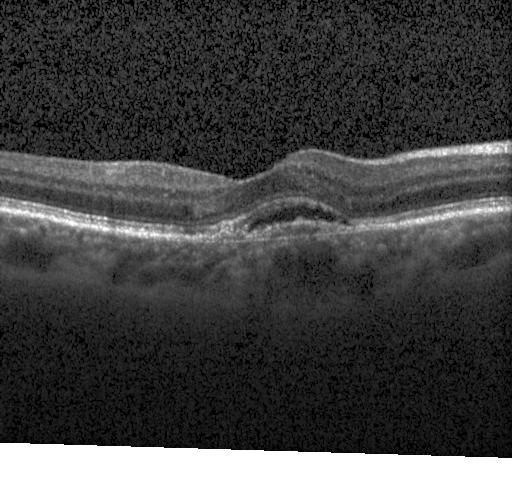 Assessment: CNV.